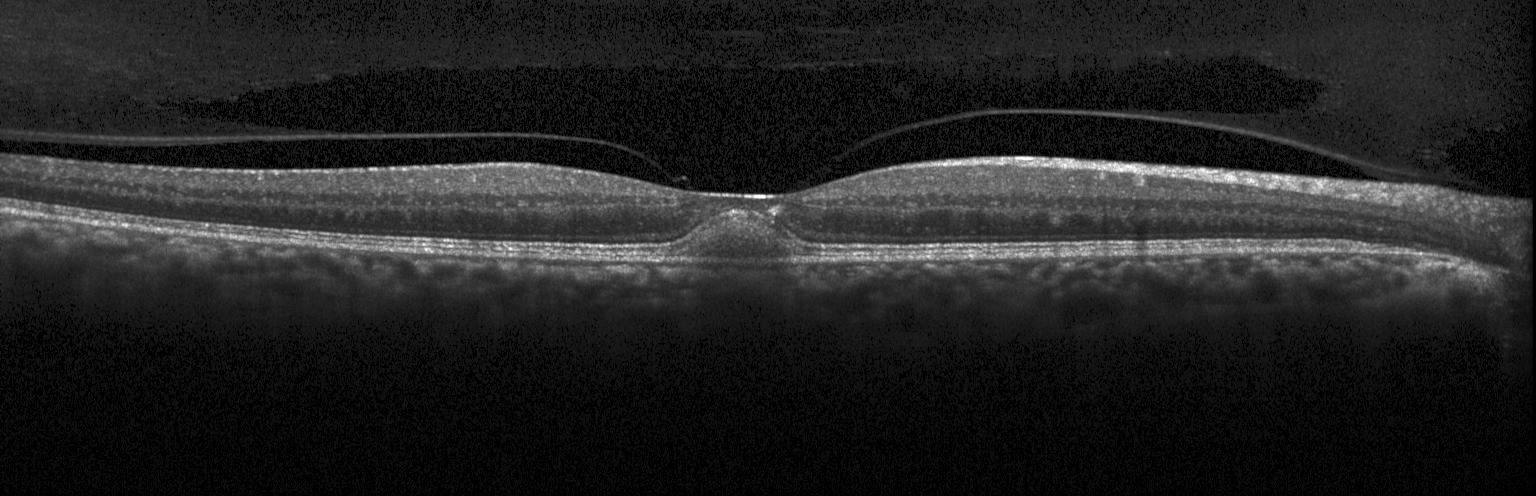

Spectral-domain optical coherence tomography. Optical coherence tomography scan — OCT finding: a choroidal neovascular membrane.